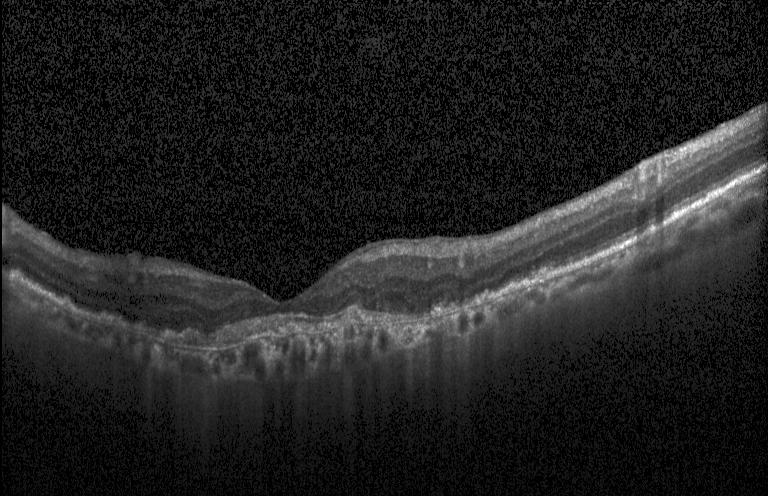

Retinal OCT cross-section · acquired on a Heidelberg Spectralis — Finding: choroidal neovascularization.